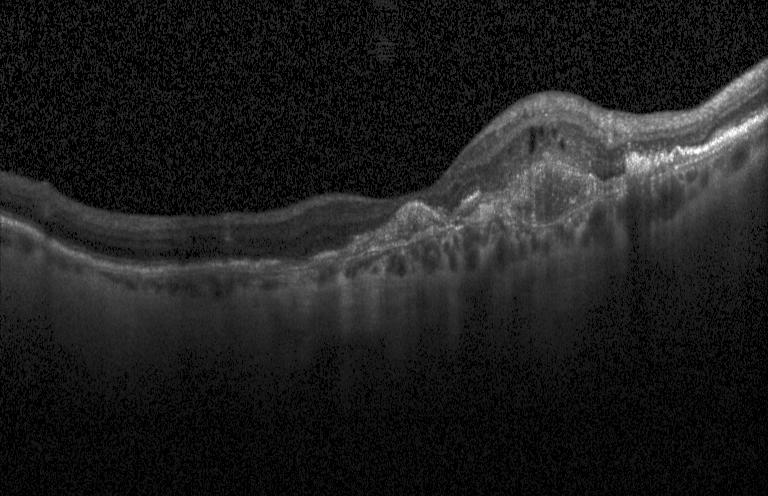

Spectral-domain OCT · retinal OCT cross-section — Impression: a choroidal neovascular membrane.